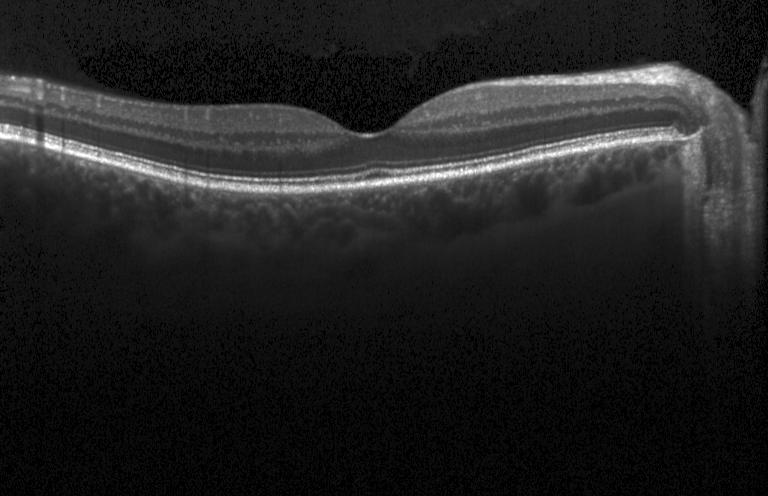

Instrument: Heidelberg Spectralis · OCT B-scan — Macular OCT: neither CNV, DME, nor drusen.